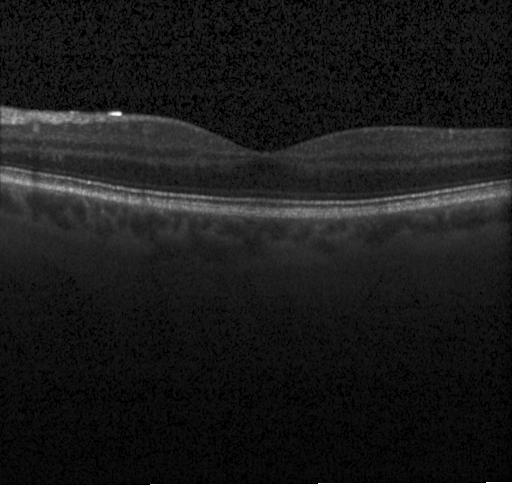
This B-scan demonstrates no choroidal neovascularization, no diabetic macular edema, and no drusen.